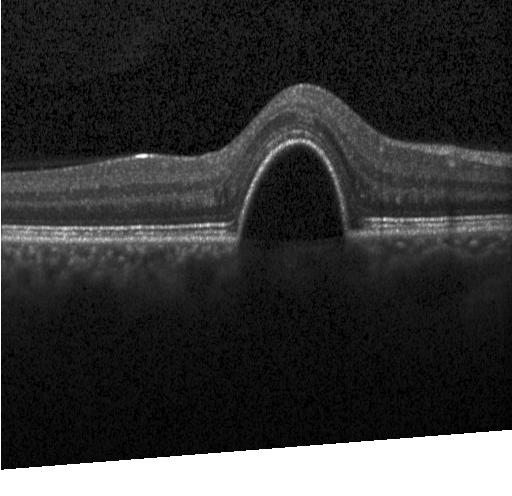

Macular scan · SD-OCT · retinal OCT B-scan · Heidelberg Spectralis — This B-scan demonstrates choroidal neovascularization.